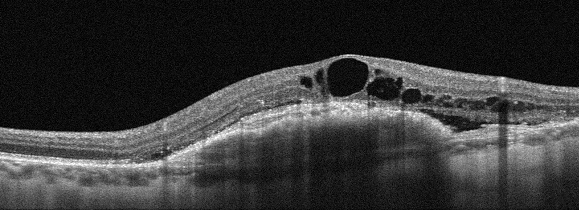

OD; retinal OCT B-scan — Dx: age-related macular degeneration (AMD).